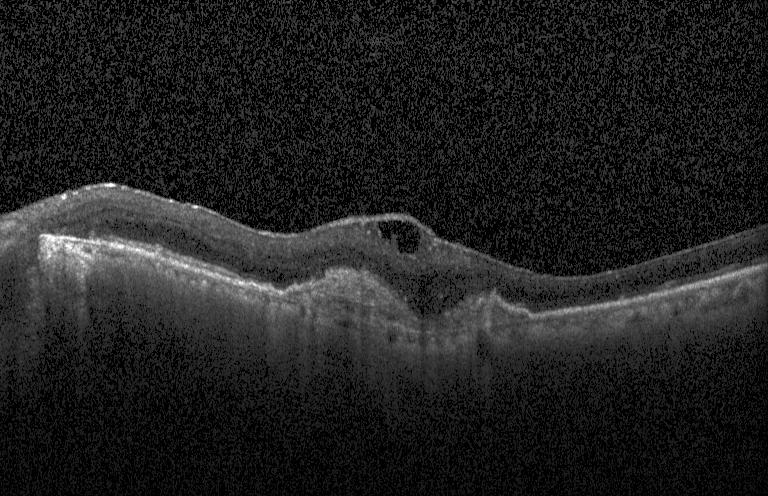

Assessment: a choroidal neovascular membrane.